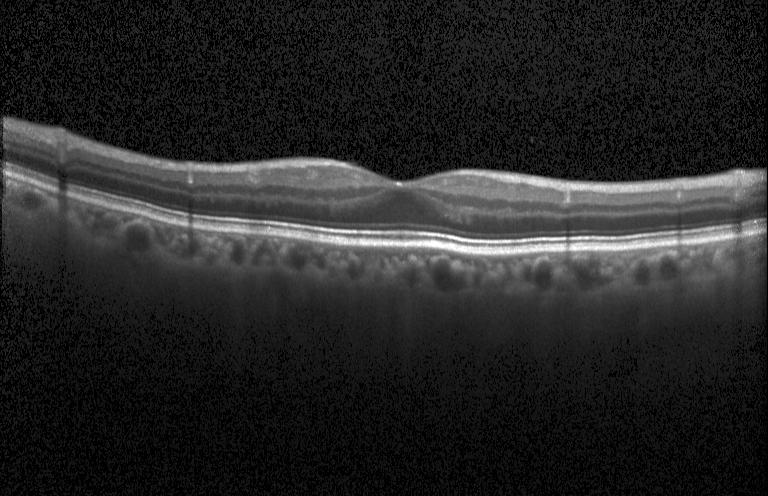
OCT B-scan showing no evidence of choroidal neovascularization, diabetic macular edema, or drusen.